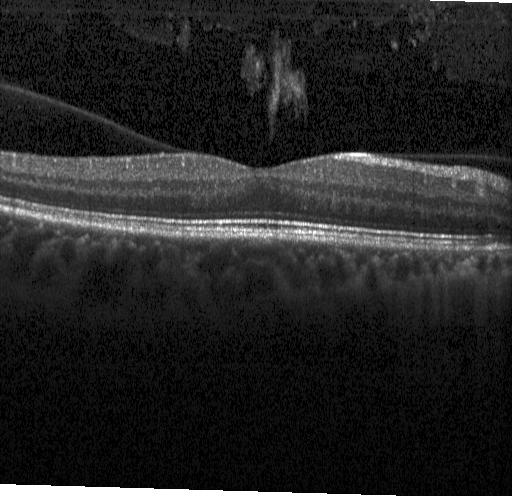

OCT B-scan. Centered on the fovea. Spectral-domain optical coherence tomography. Impression: no choroidal neovascularization, no diabetic macular edema, and no drusen.